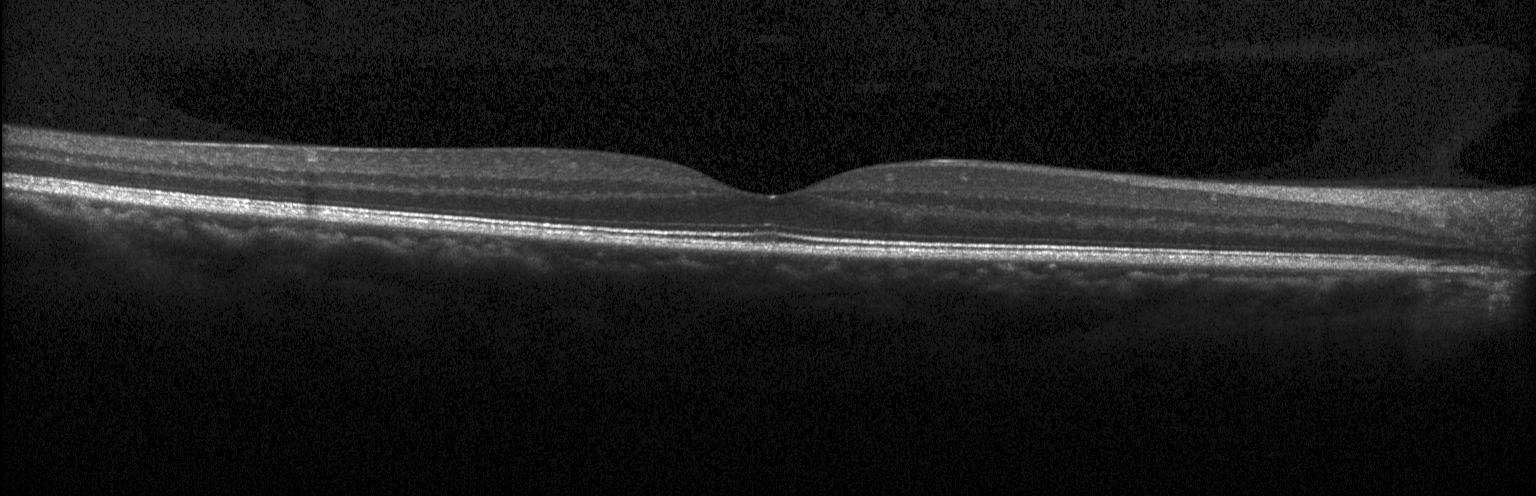 Spectral-domain OCT, centered on the fovea, OCT B-scan, Heidelberg Spectralis OCT system. Impression: no CNV, no DME, and no drusen.